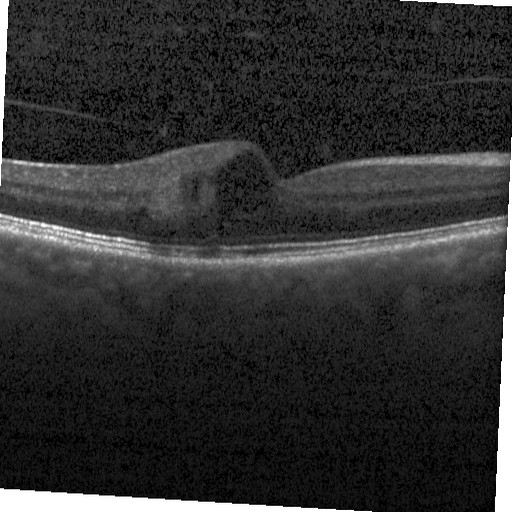 The scan shows diabetic macular edema.